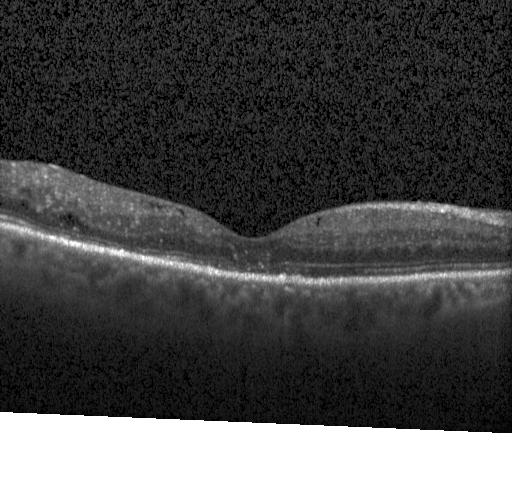 OCT finding: DME.